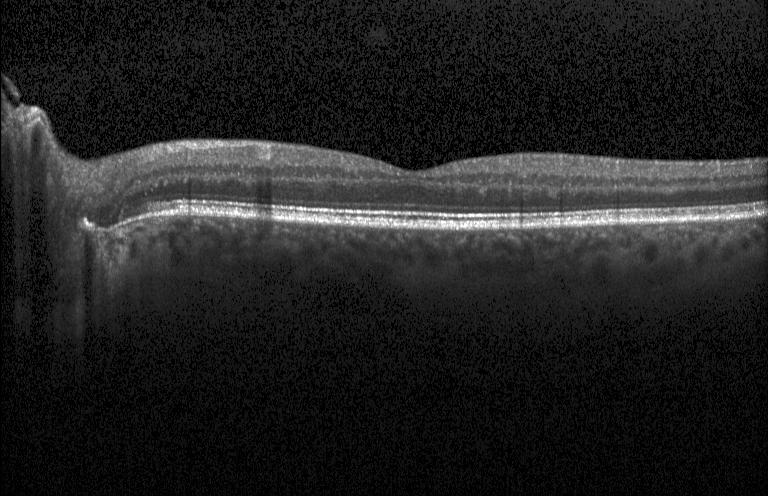

Retinal OCT cross-section showing no CNV, DME, or drusen.